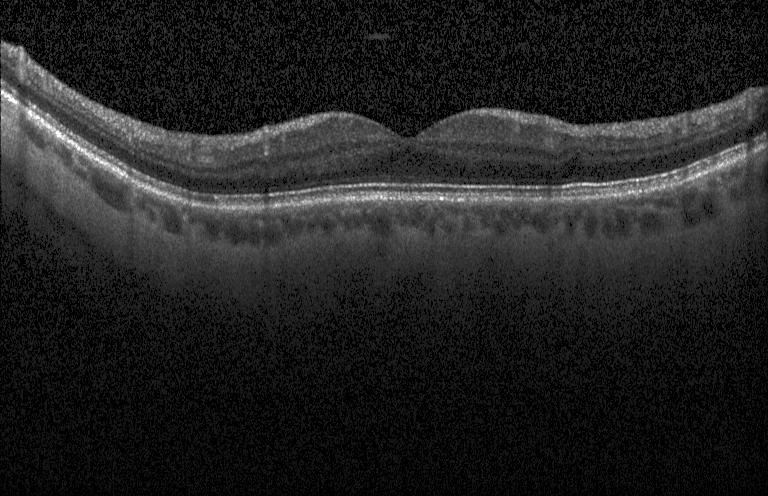
SD-OCT · macular scan · Heidelberg Spectralis OCT system · OCT line scan
Diagnosis: no evidence of choroidal neovascularization, diabetic macular edema, or drusen.